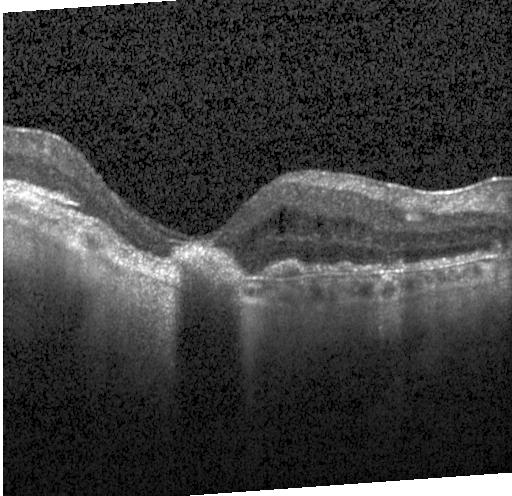

Spectral-domain OCT B-scan: choroidal neovascularization.